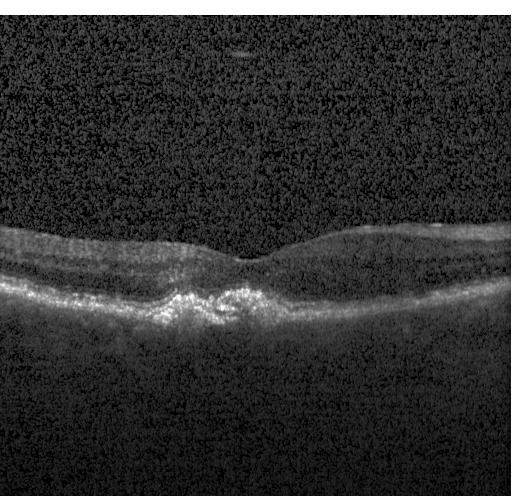
Impression: choroidal neovascularization.